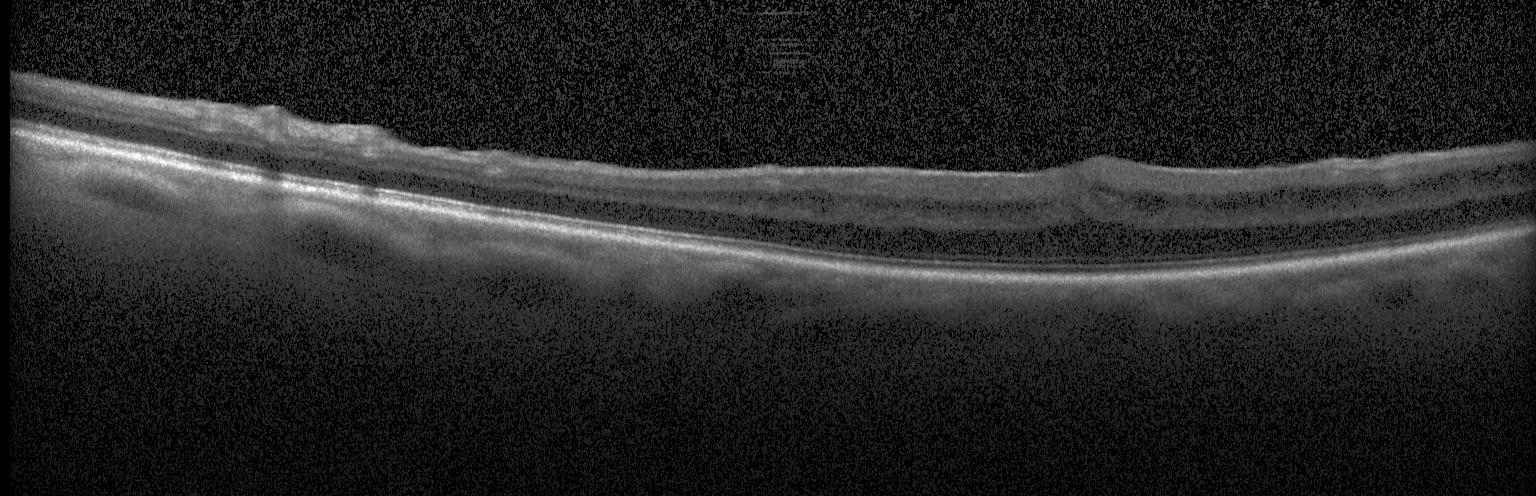

Horizontal scan through the fovea, instrument: Heidelberg Spectralis, retinal OCT cross-section
Finding: diabetic macular edema (DME).